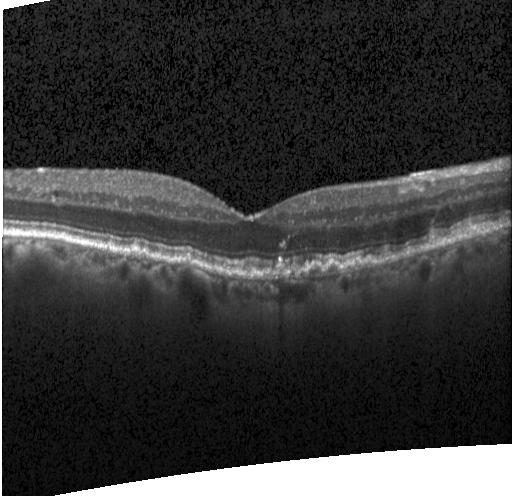

Spectral-domain OCT B-scan: sub-RPE drusenoid deposits.